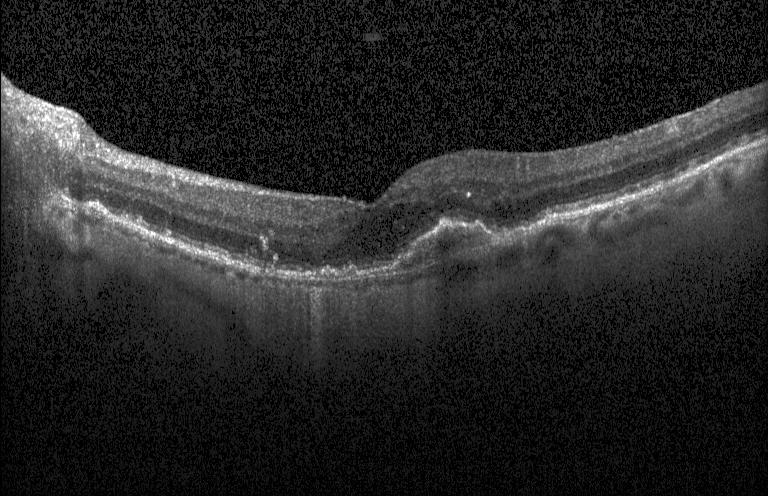

Assessment: CNV.